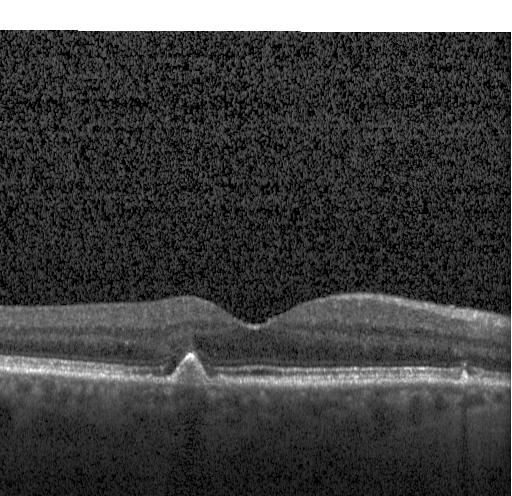
Fovea-centered, retinal OCT cross-section — Multiple drusen.